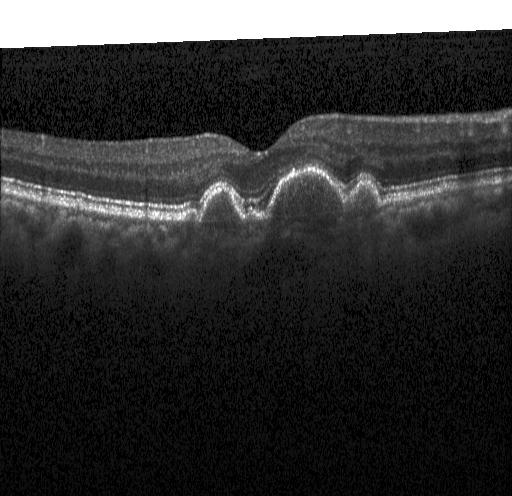
OCT B-scan · Heidelberg Spectralis OCT system — OCT finding: multiple drusen.